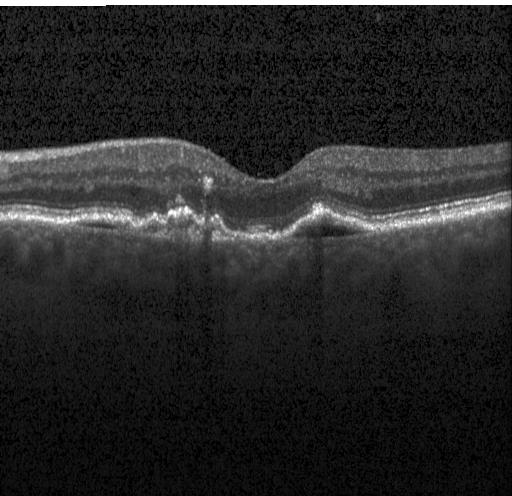

OCT B-scan showing choroidal neovascularization (CNV).